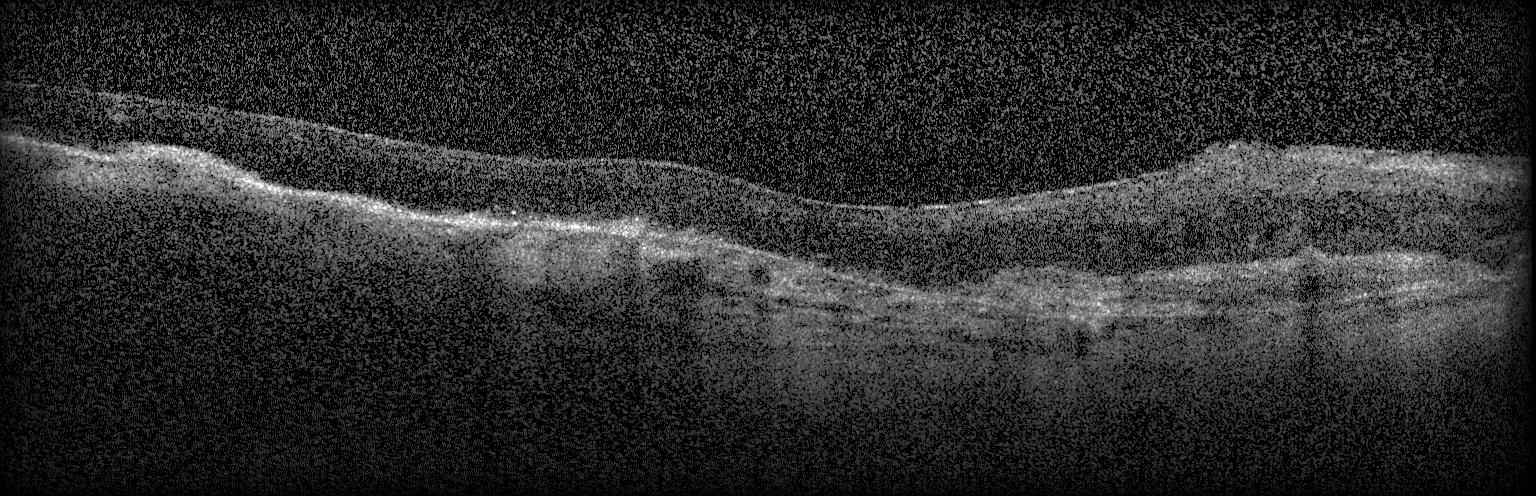

Impression: a choroidal neovascular membrane.